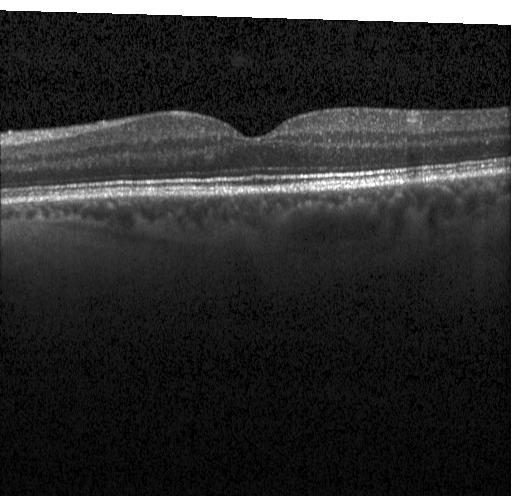

Spectral-domain OCT · through the macula · retinal OCT cross-section. Impression: no CNV, DME, or drusen.